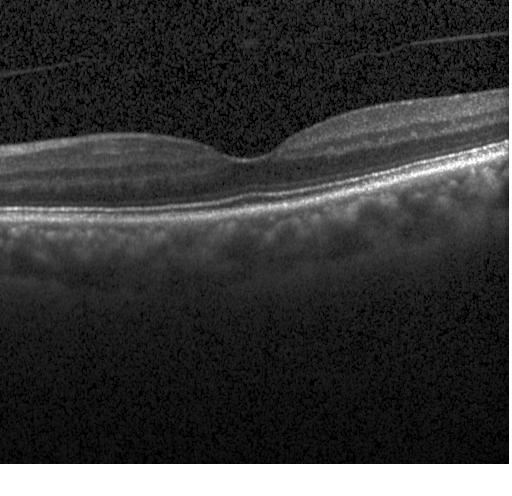

SD-OCT, optical coherence tomography scan, macular scan, Heidelberg Spectralis OCT system. This B-scan demonstrates no choroidal neovascularization, diabetic macular edema, or drusen.